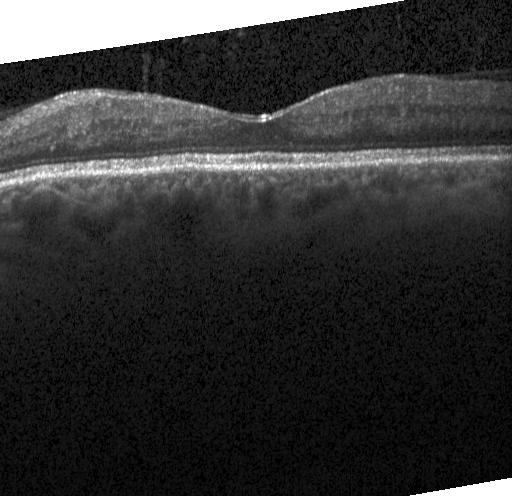 Finding: neither CNV, DME, nor drusen.